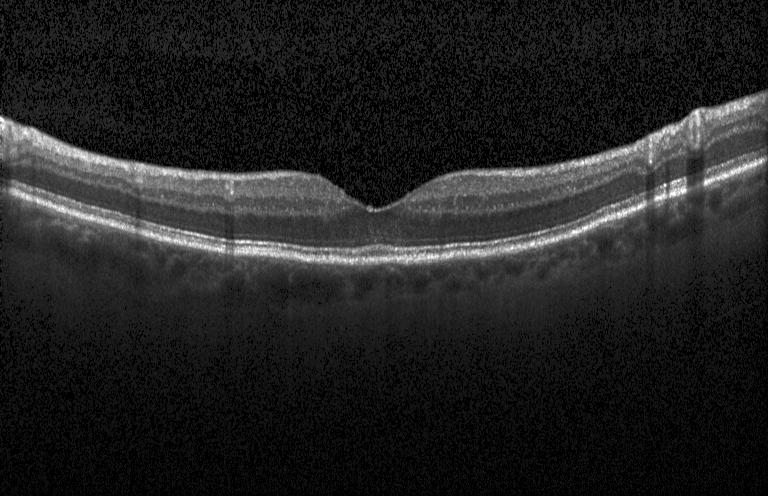

Finding: no choroidal neovascularization, diabetic macular edema, or drusen.